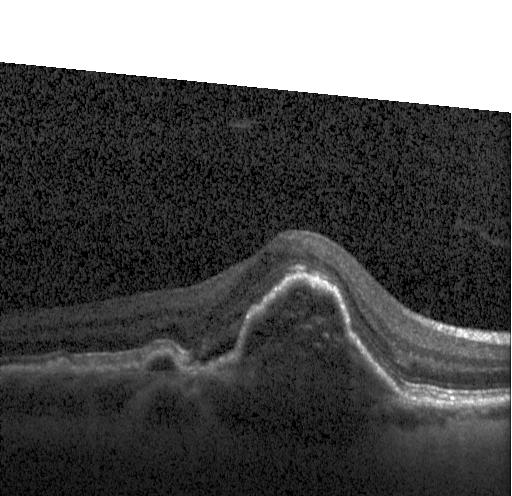 Optical coherence tomography B-scan. Macular scan
This B-scan demonstrates choroidal neovascularization (CNV).